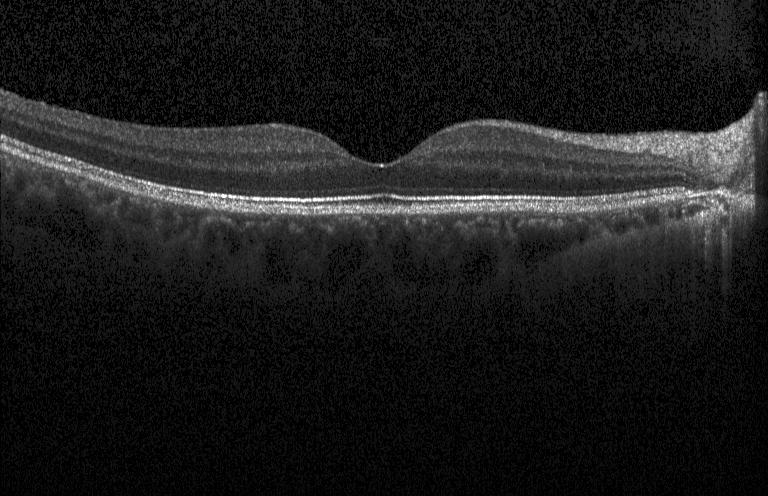

Spectral-domain optical coherence tomography, acquired on a Heidelberg Spectralis, retinal OCT B-scan — This B-scan demonstrates neither choroidal neovascularization, diabetic macular edema, nor drusen.